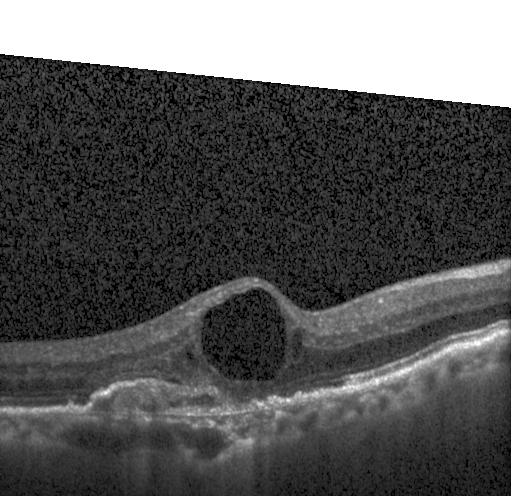

Instrument: Heidelberg Spectralis. Retinal OCT cross-section. Spectral-domain optical coherence tomography. Through the macula. Diagnosis: a choroidal neovascular membrane.